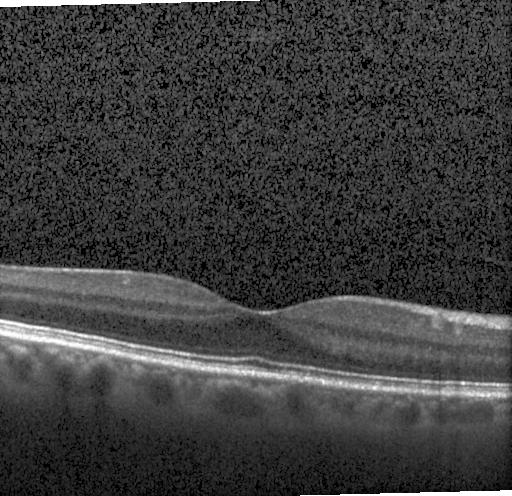
OCT B-scan showing no choroidal neovascularization, diabetic macular edema, or drusen.